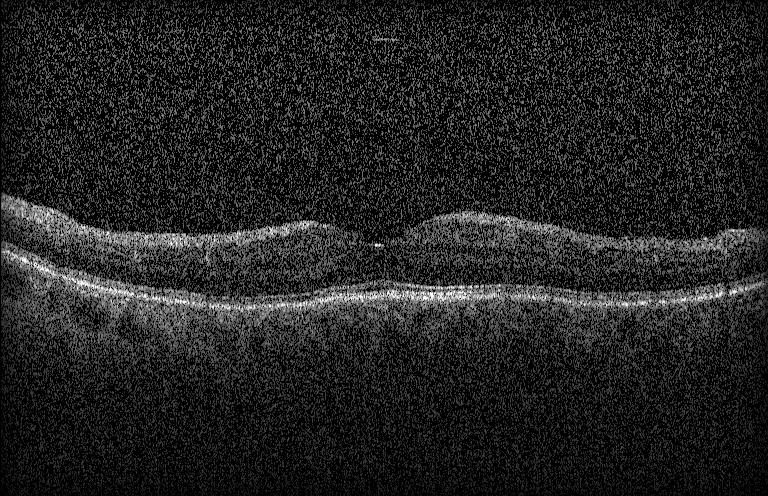 OCT B-scan, Heidelberg Spectralis, macular scan, SD-OCT — Impression: no choroidal neovascularization, diabetic macular edema, or drusen.